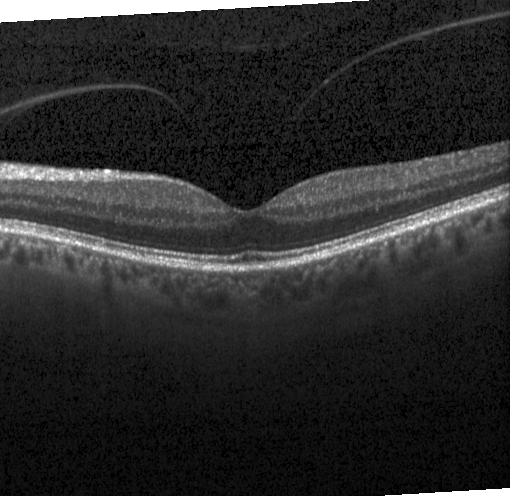

OCT line scan.
Finding: no choroidal neovascularization, no diabetic macular edema, and no drusen.